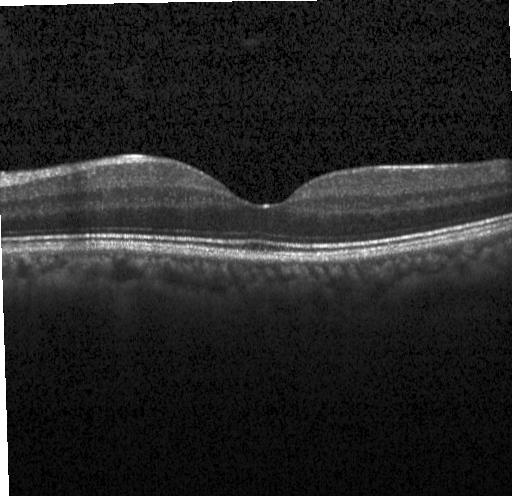
Optical coherence tomography scan. Macular scan. SD-OCT. Acquired on a Heidelberg Spectralis
This B-scan demonstrates no choroidal neovascularization, diabetic macular edema, or drusen.